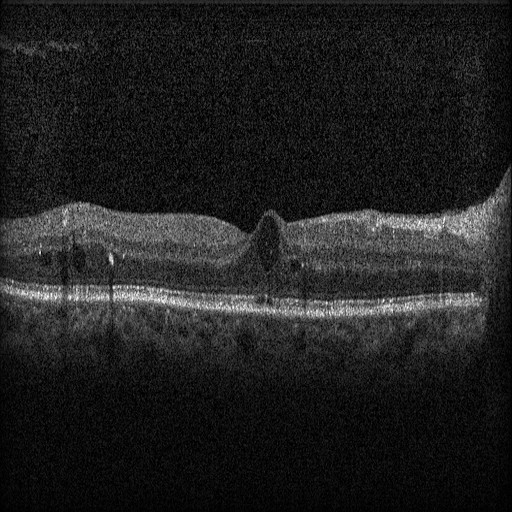
Centered on the fovea; retinal OCT cross-section; Heidelberg Spectralis OCT system
Macular OCT: diabetic macular edema.